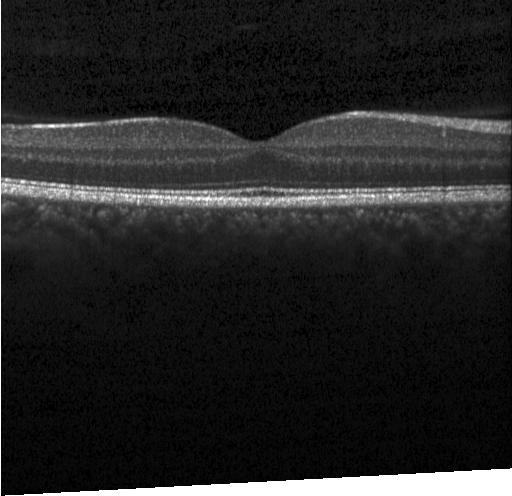 OCT line scan. SD-OCT. Instrument: Heidelberg Spectralis. Fovea-centered.
Impression: neither choroidal neovascularization, diabetic macular edema, nor drusen.